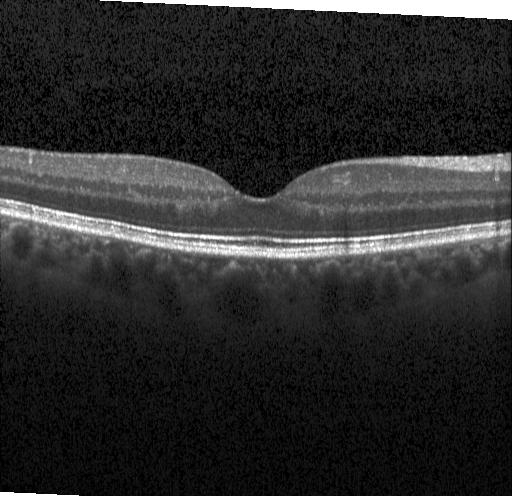

Diagnosis: no choroidal neovascularization, diabetic macular edema, or drusen.